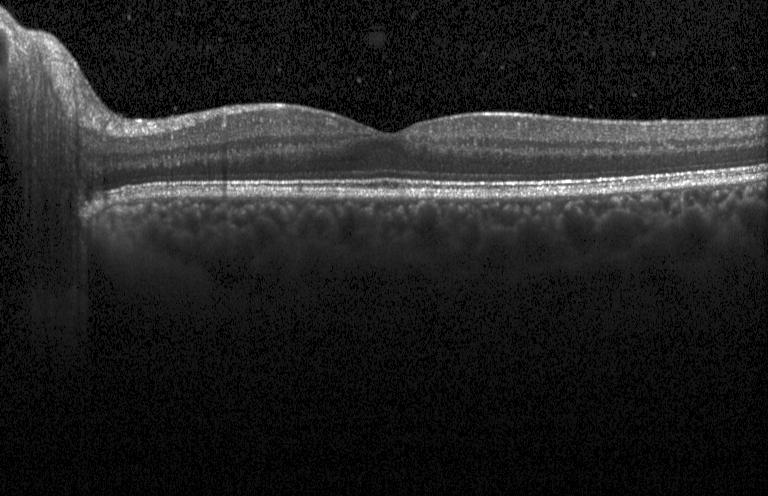 OCT line scan. Finding: no choroidal neovascularization, diabetic macular edema, or drusen.